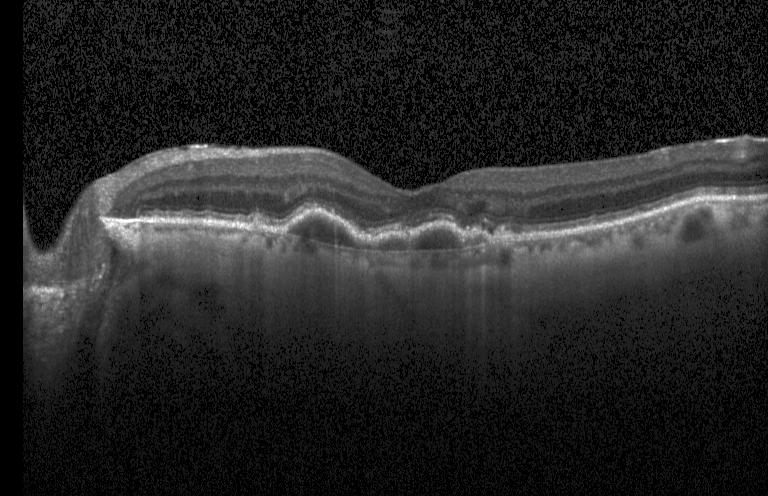 OCT B-scan — Macular OCT: choroidal neovascularization.